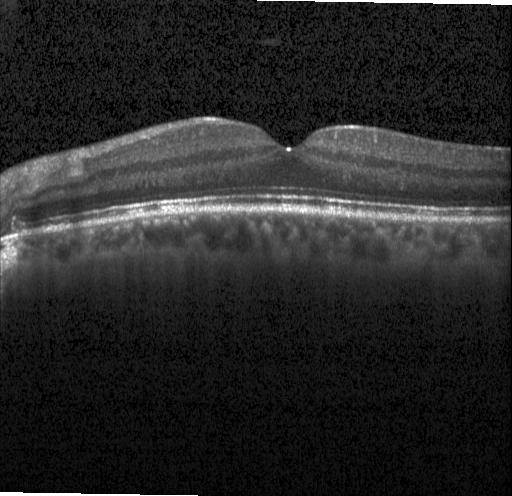

The scan shows neither CNV, DME, nor drusen.